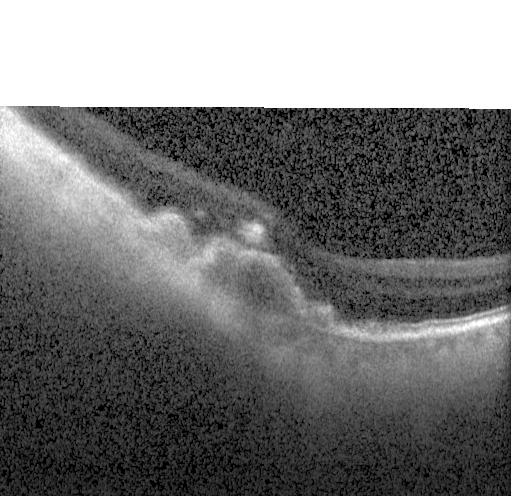
Assessment: choroidal neovascularization (CNV).